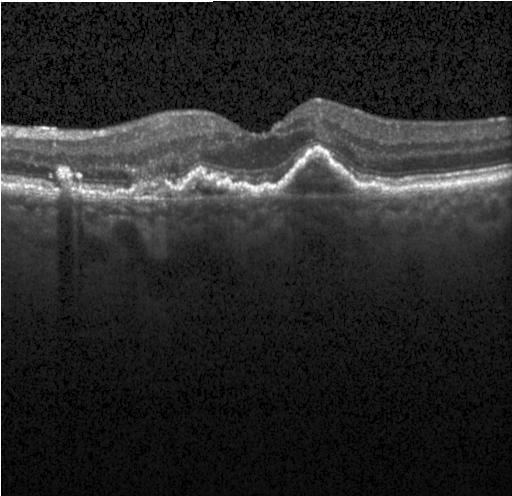
Centered on the fovea. SD-OCT. Optical coherence tomography B-scan.
A choroidal neovascular membrane.